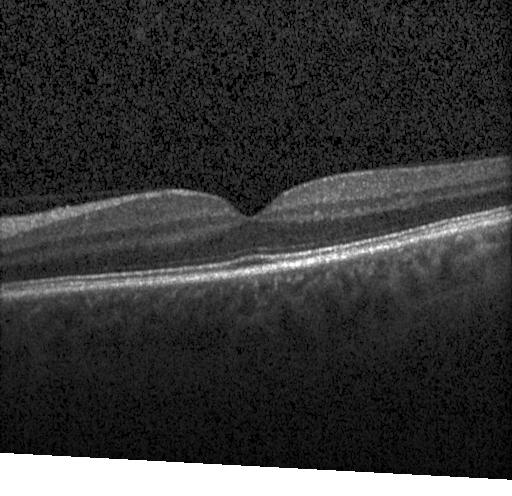
Heidelberg Spectralis OCT system; optical coherence tomography scan. Dx: no evidence of choroidal neovascularization, diabetic macular edema, or drusen.